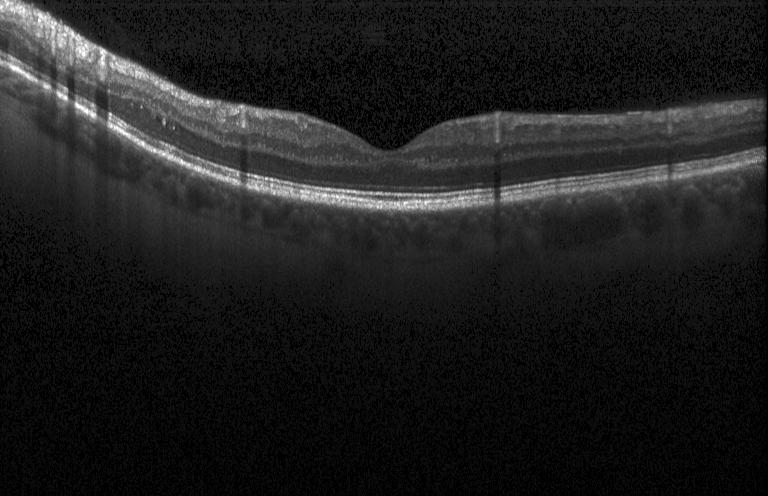 OCT B-scan — Finding: no choroidal neovascularization, diabetic macular edema, or drusen.